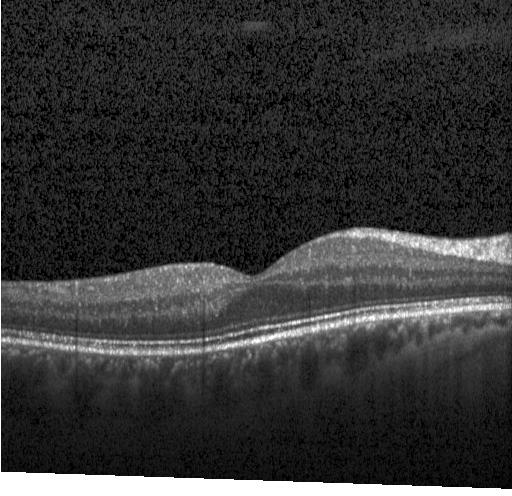
OCT B-scan showing no choroidal neovascularization, no diabetic macular edema, and no drusen.